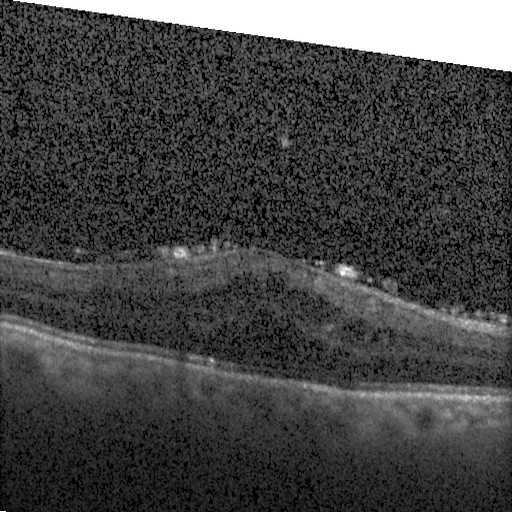 Horizontal scan through the fovea; optical coherence tomography B-scan; SD-OCT; Heidelberg Spectralis. DME.